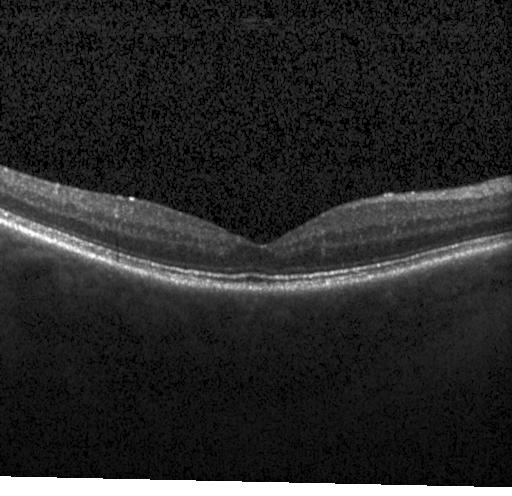
OCT finding: no choroidal neovascularization, no diabetic macular edema, and no drusen.